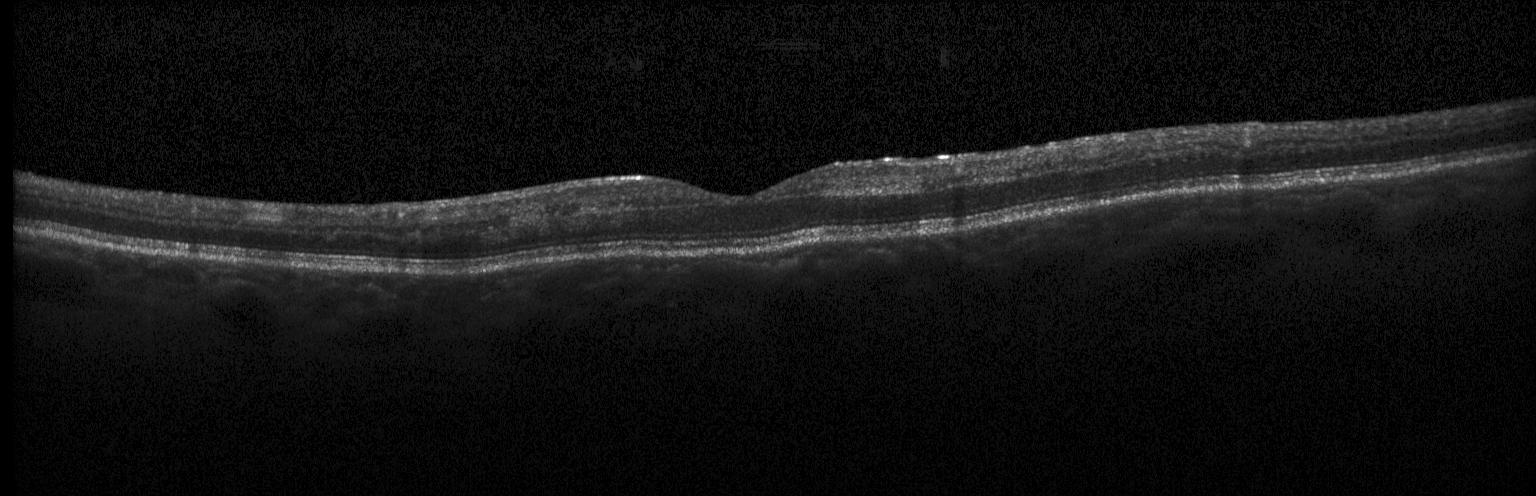 Diagnosis: no choroidal neovascularization, diabetic macular edema, or drusen.